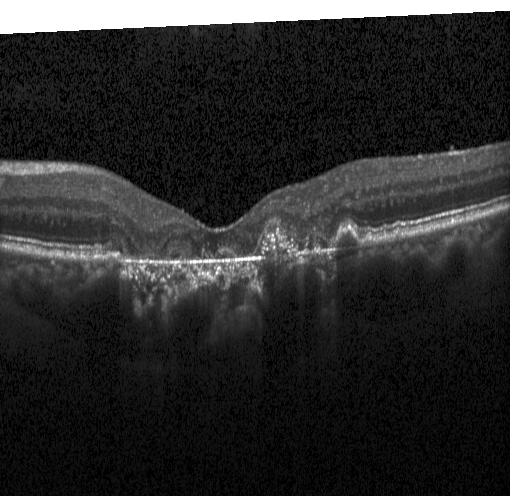 OCT scan showing a choroidal neovascular membrane.